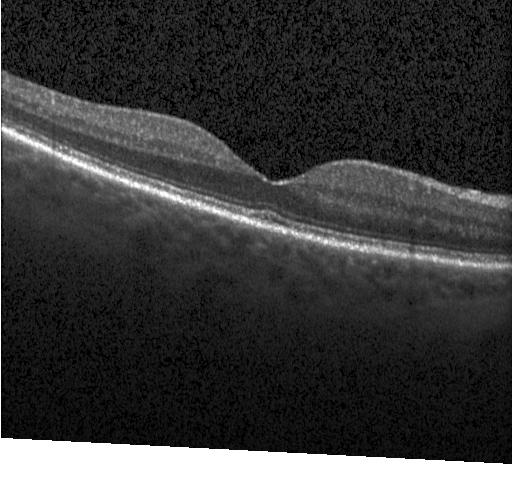

Dx: no evidence of choroidal neovascularization, diabetic macular edema, or drusen.